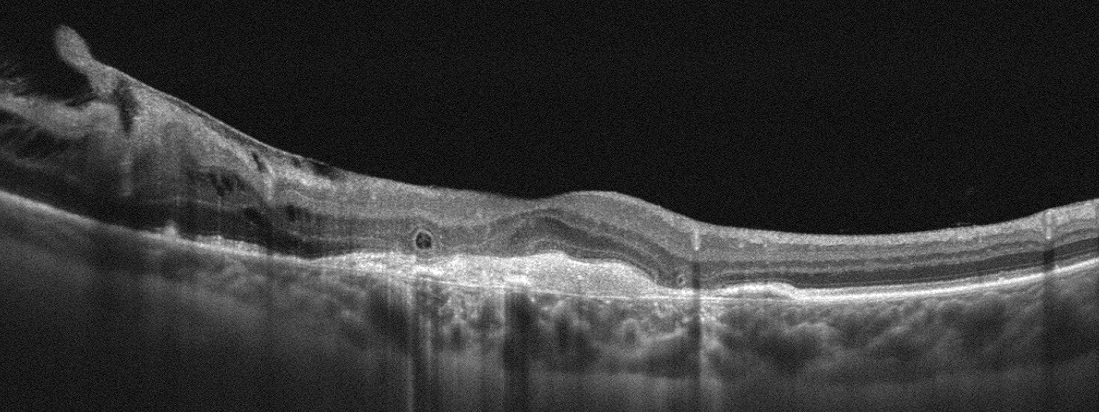

OCT B-scan showing AMD.